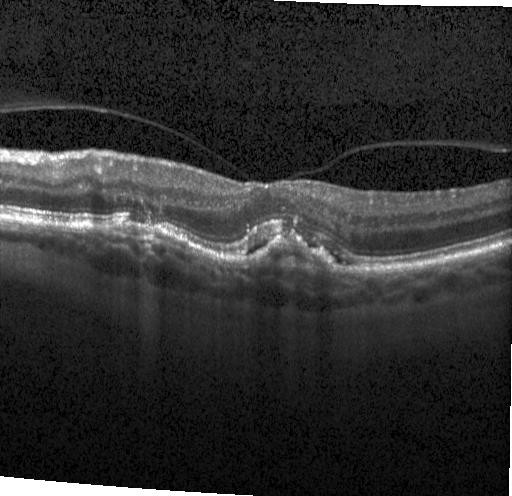 Spectral-domain OCT; OCT B-scan — The scan shows a choroidal neovascular membrane.